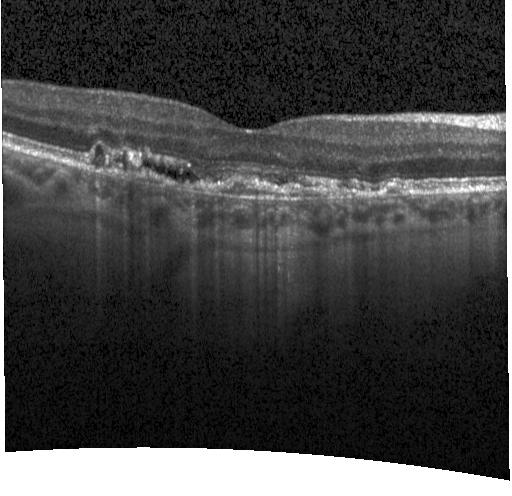 OCT B-scan showing CNV.